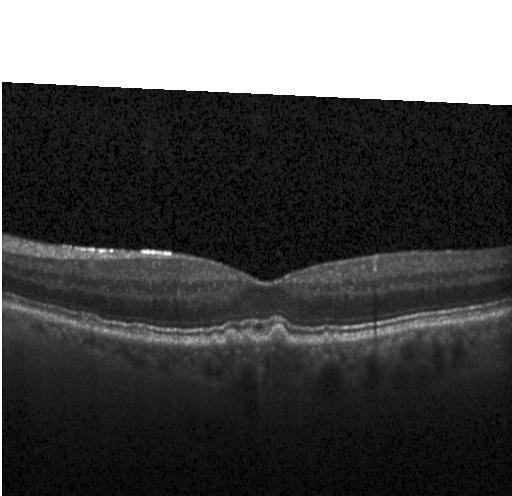

Spectral-domain OCT B-scan: sub-RPE drusenoid deposits.